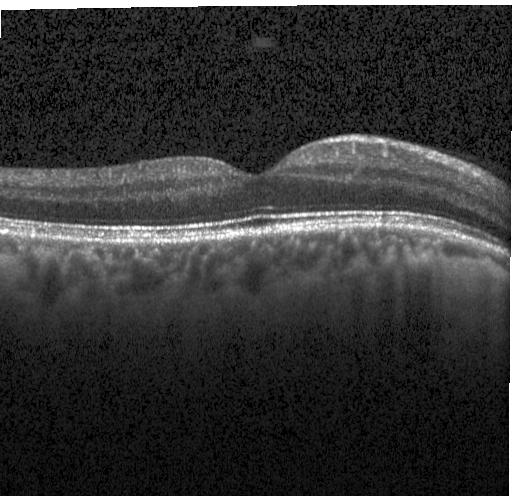 Retinal OCT cross-section; acquired on a Heidelberg Spectralis; through the macula — Finding: no evidence of CNV, DME, or drusen.